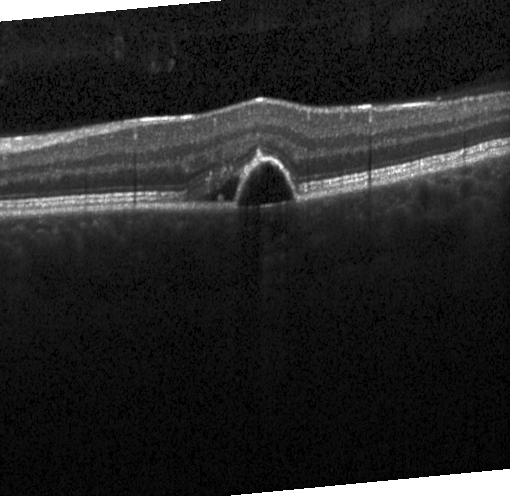 The scan shows CNV.